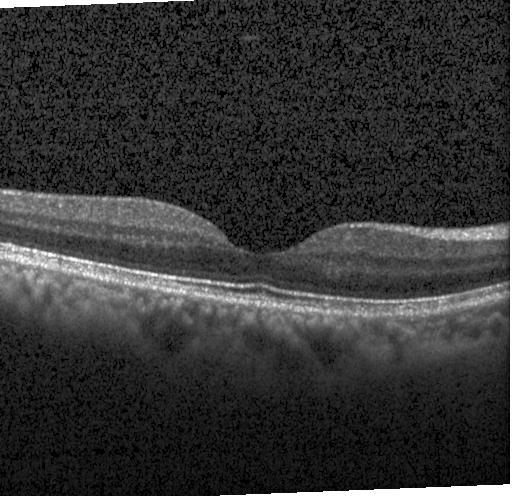

OCT B-scan showing neither CNV, DME, nor drusen.